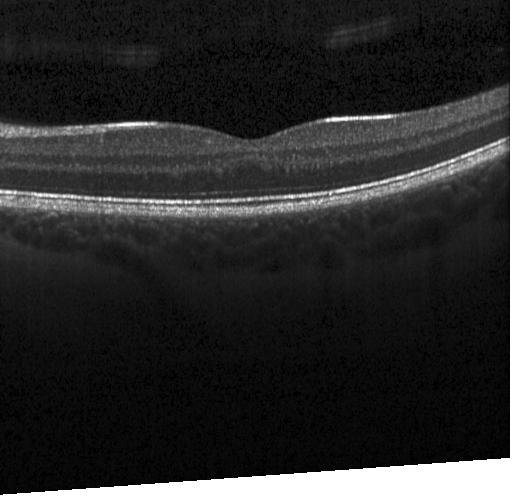

Diagnosis: neither choroidal neovascularization, diabetic macular edema, nor drusen.